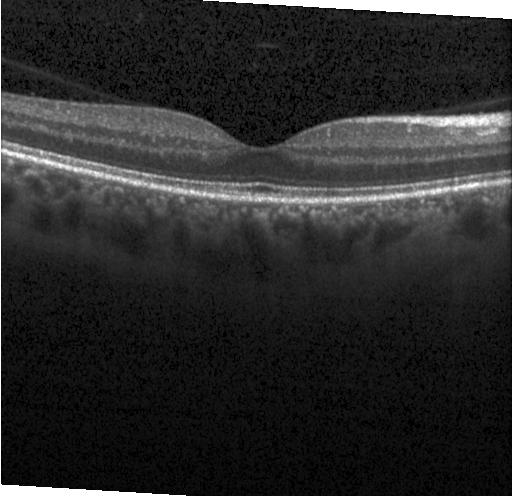

Through the macula, optical coherence tomography scan, Heidelberg Spectralis OCT system, spectral-domain OCT. No evidence of choroidal neovascularization, diabetic macular edema, or drusen.